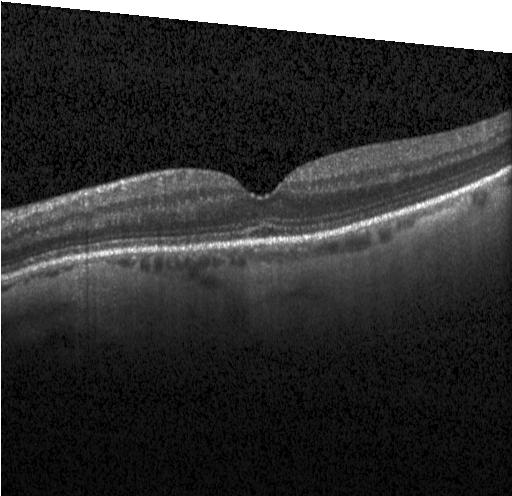
Heidelberg Spectralis, OCT B-scan.
Finding: neither choroidal neovascularization, diabetic macular edema, nor drusen.